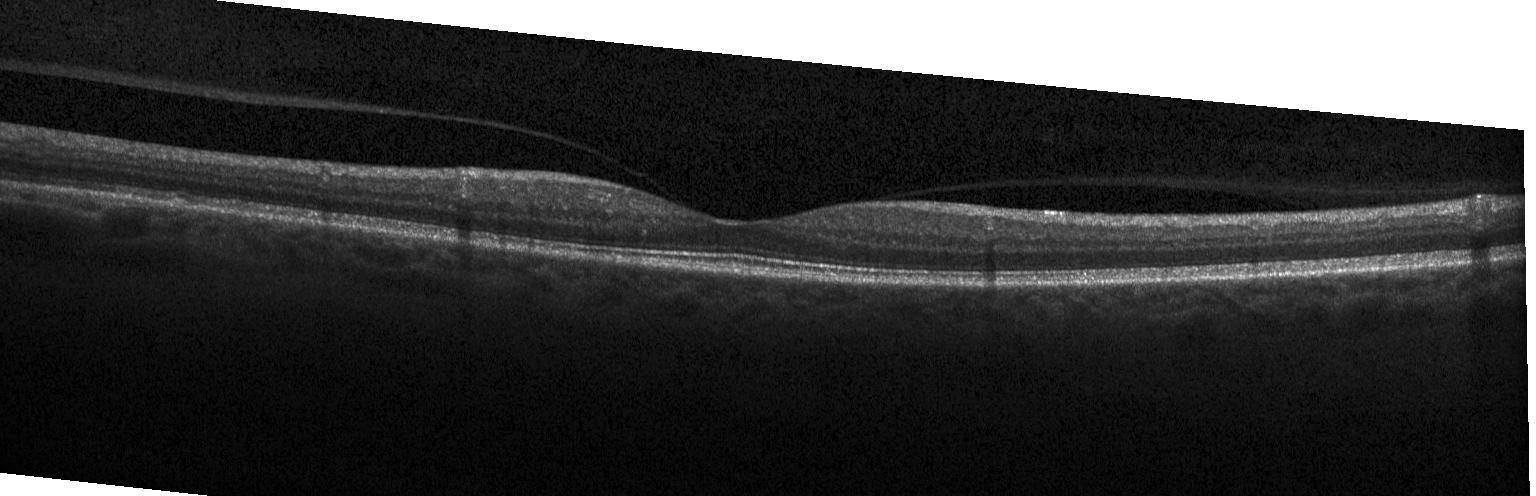 Finding: neither choroidal neovascularization, diabetic macular edema, nor drusen.